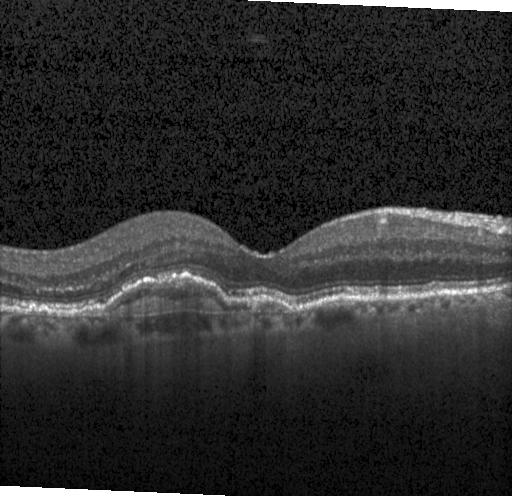

Heidelberg Spectralis · SD-OCT · OCT line scan · fovea-centered.
Diagnosis: a choroidal neovascular membrane.